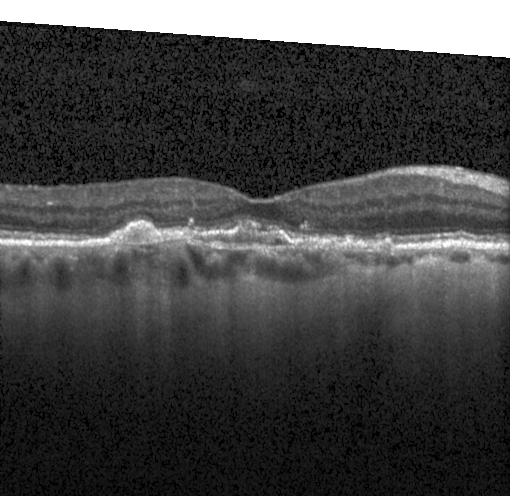 Optical coherence tomography scan
This B-scan demonstrates choroidal neovascularization.